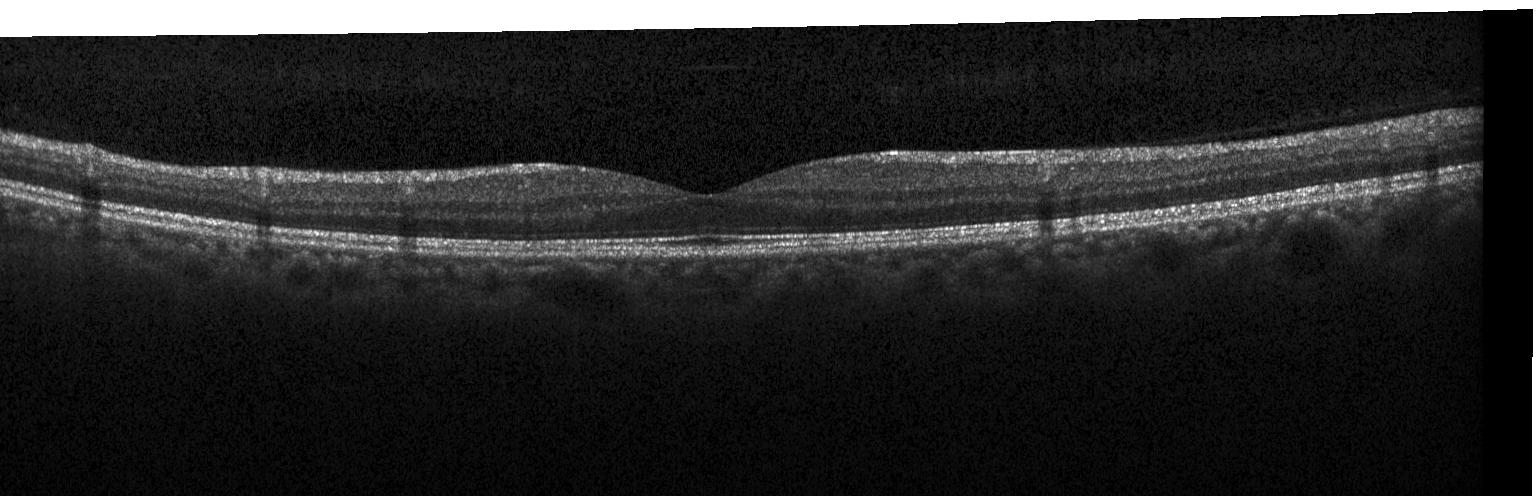
Retinal OCT cross-section, Heidelberg Spectralis OCT system.
The scan shows neither choroidal neovascularization, diabetic macular edema, nor drusen.